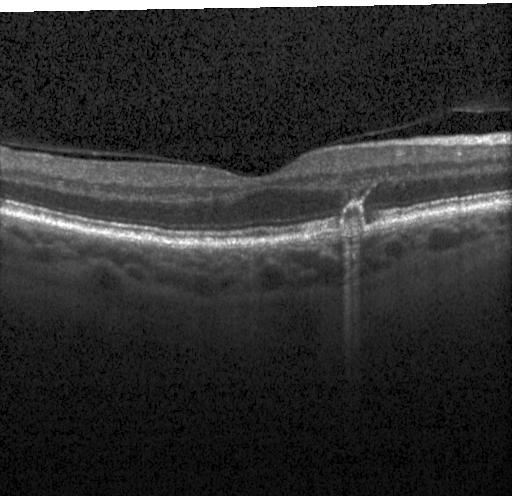

OCT line scan; macular scan.
Sub-RPE drusenoid deposits.